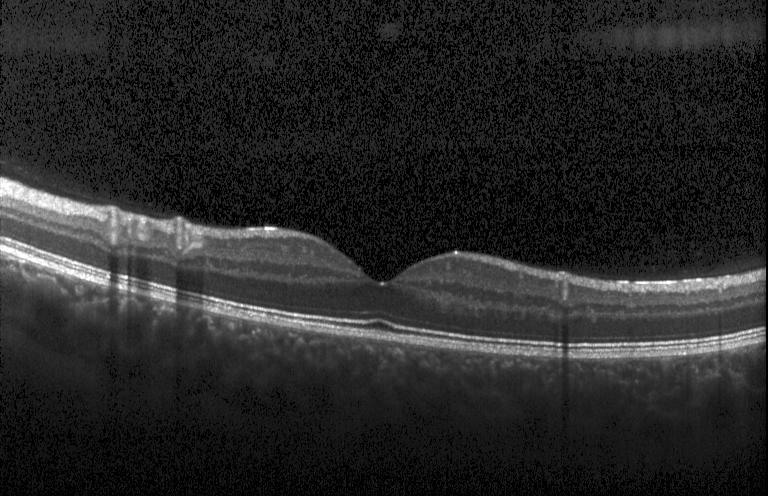
Spectral-domain OCT. OCT B-scan.
This B-scan demonstrates no CNV, DME, or drusen.